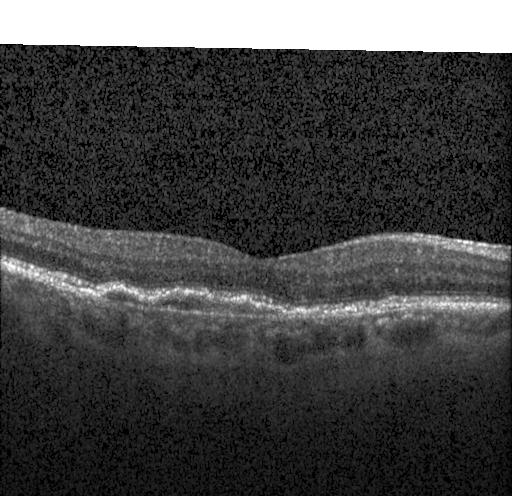 Diagnosis: a choroidal neovascular membrane.